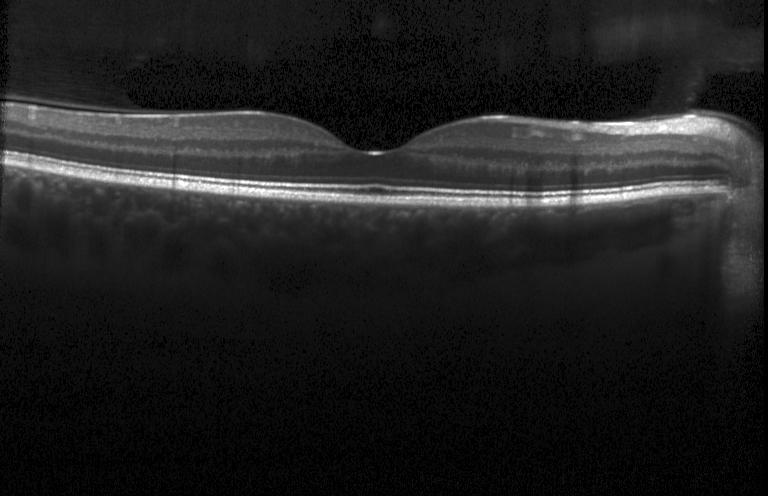
Optical coherence tomography B-scan. Spectral-domain OCT. Acquired on a Heidelberg Spectralis. Through the macula. Dx: no CNV, DME, or drusen.